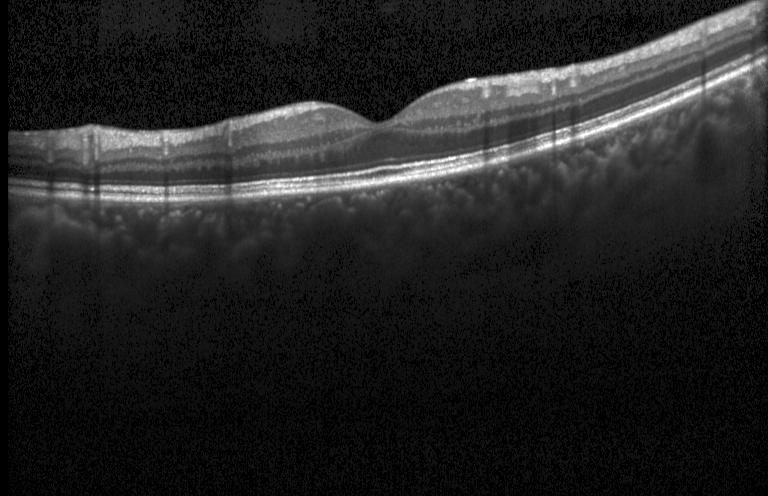
OCT finding: no CNV, no DME, and no drusen.